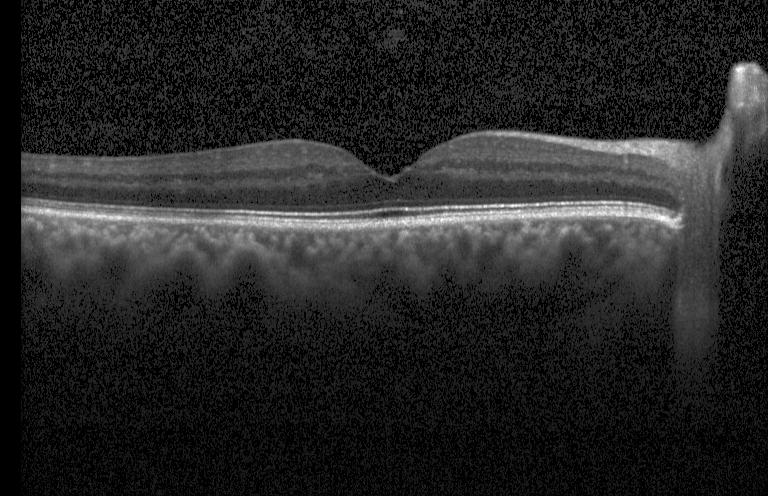

Macular scan; Heidelberg Spectralis; retinal OCT B-scan.
Assessment: no evidence of choroidal neovascularization, diabetic macular edema, or drusen.